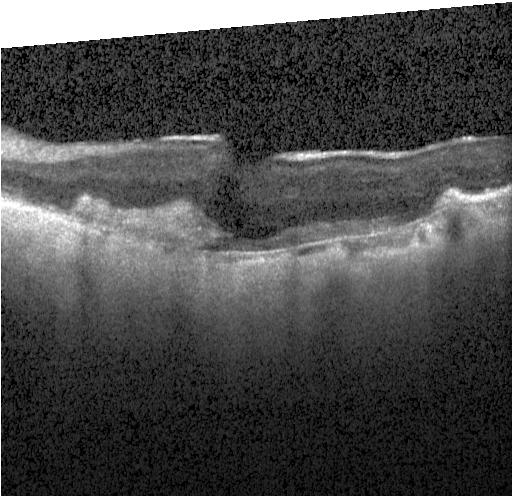
Optical coherence tomography B-scan — This B-scan demonstrates a choroidal neovascular membrane.